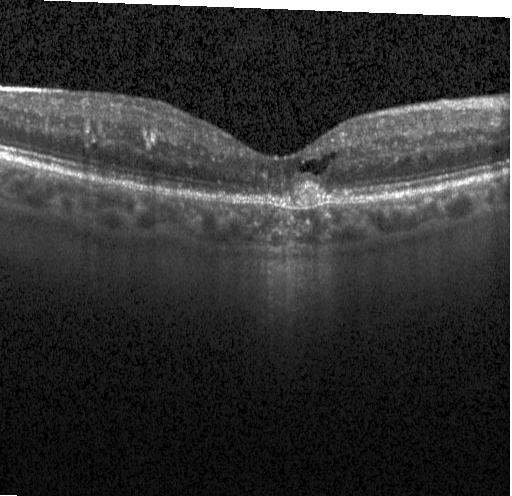
Retinal OCT B-scan; Heidelberg Spectralis; through the macula — Macular OCT: choroidal neovascularization.